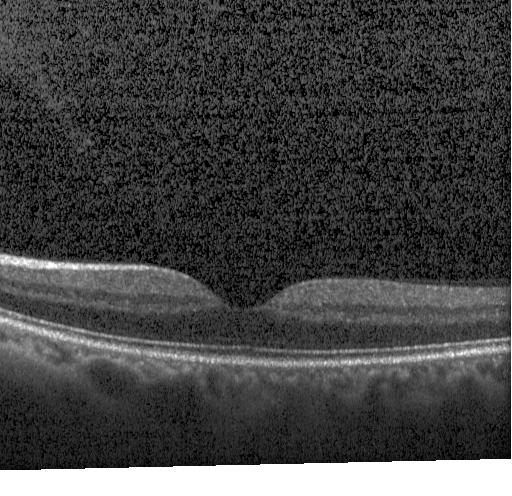
Macular scan, Heidelberg Spectralis OCT system, retinal OCT cross-section. Impression: no choroidal neovascularization, diabetic macular edema, or drusen.